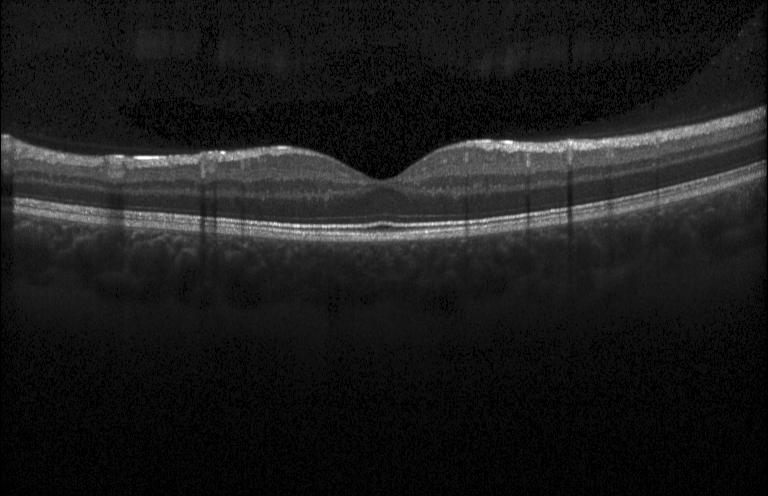
Impression: no evidence of CNV, DME, or drusen.